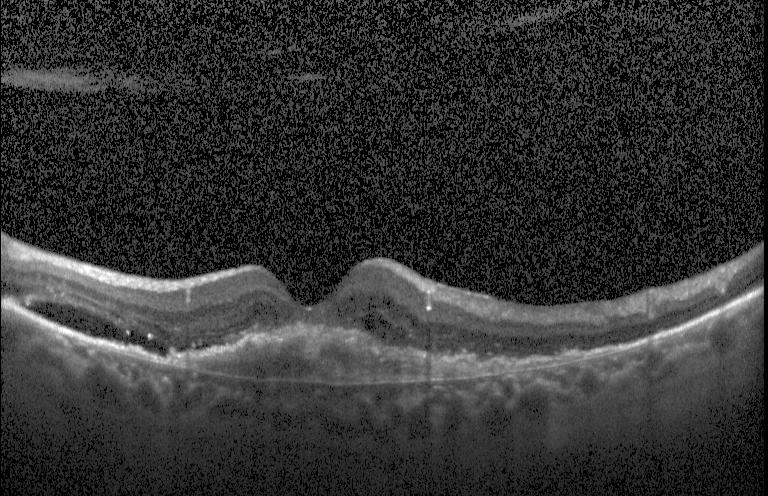
Retinal OCT cross-section · macular scan.
Finding: a choroidal neovascular membrane.